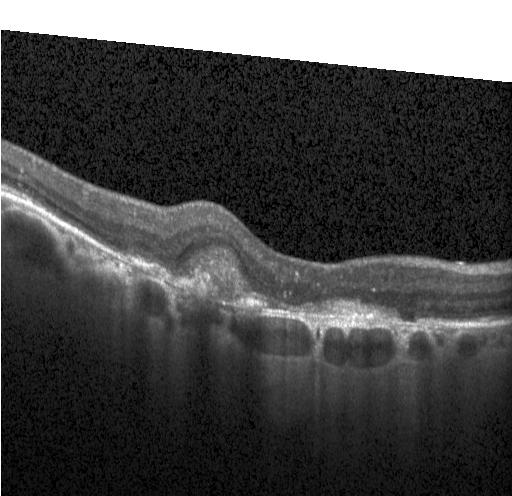

Spectral-domain OCT, Heidelberg Spectralis, OCT B-scan, fovea-centered — Finding: a choroidal neovascular membrane.